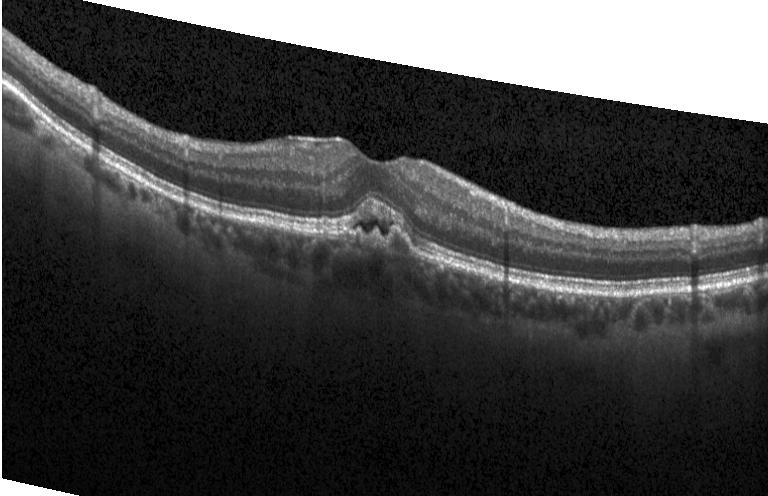 Dx: a choroidal neovascular membrane.